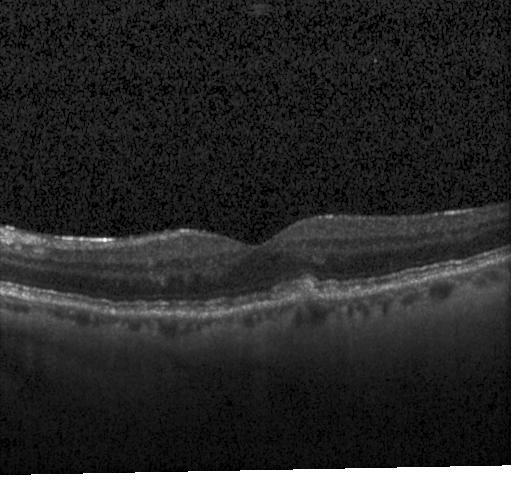

Macular OCT demonstrating multiple drusen.